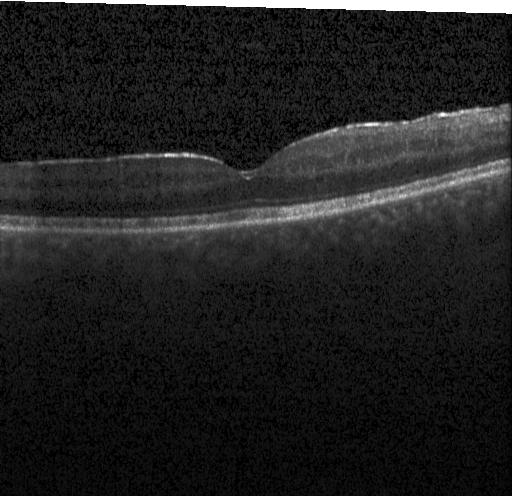 Through the macula · retinal OCT cross-section · spectral-domain optical coherence tomography · Heidelberg Spectralis OCT system — OCT finding: no evidence of choroidal neovascularization, diabetic macular edema, or drusen.